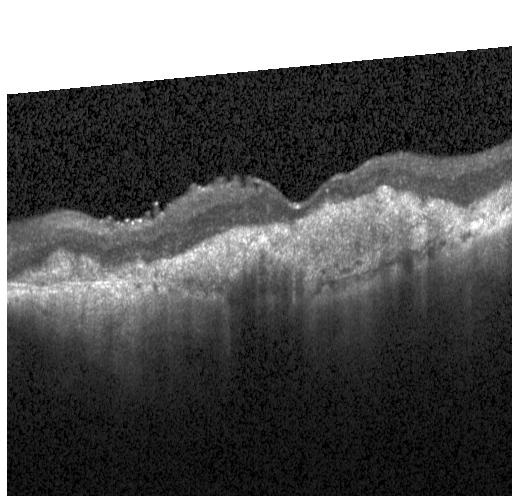
Horizontal scan through the fovea. Retinal OCT B-scan. Spectral-domain optical coherence tomography. Instrument: Heidelberg Spectralis
Finding: CNV.